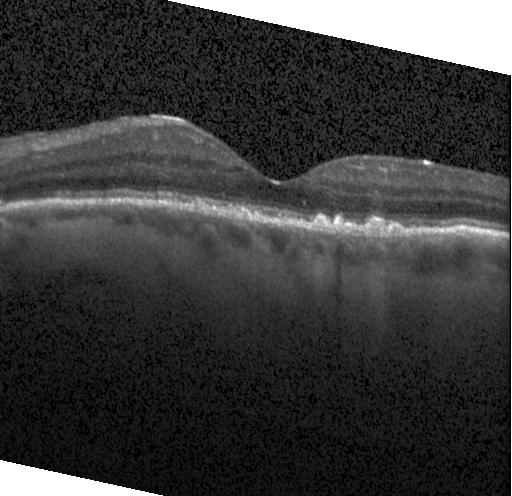

Spectral-domain optical coherence tomography · retinal OCT B-scan — The scan shows multiple drusen.